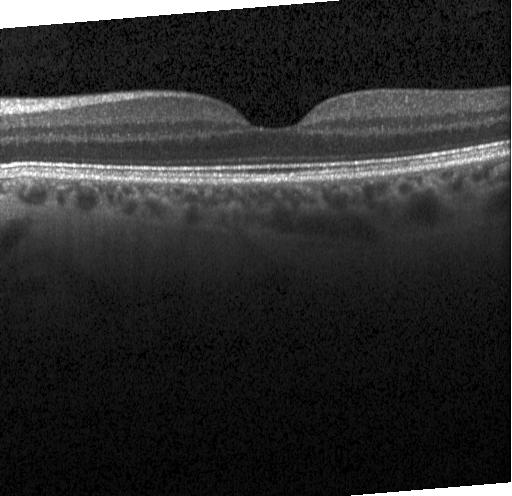
Finding: no evidence of CNV, DME, or drusen.